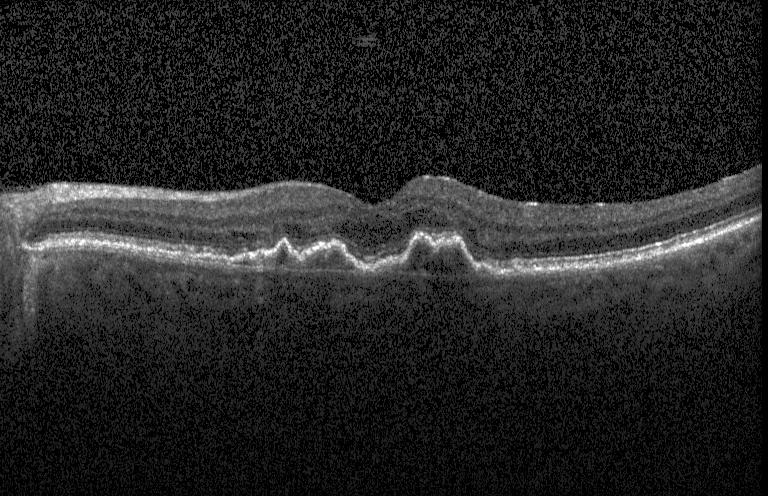 Retinal OCT cross-section
This B-scan demonstrates a choroidal neovascular membrane.